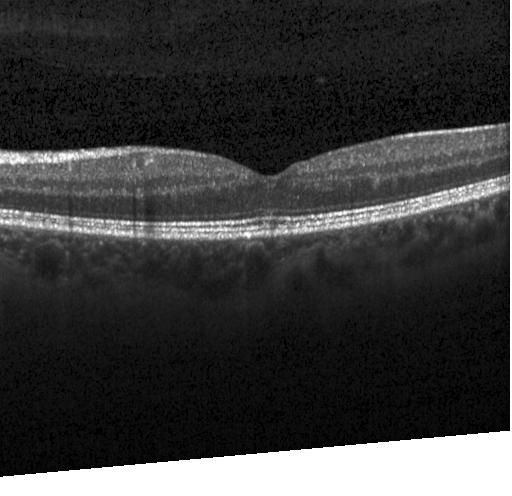

Macular scan. Spectral-domain OCT. Retinal OCT B-scan.
Impression: no evidence of choroidal neovascularization, diabetic macular edema, or drusen.